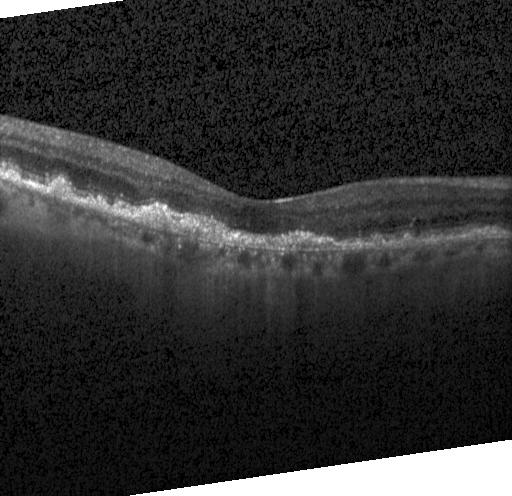
Retinal OCT B-scan, fovea-centered.
A choroidal neovascular membrane.